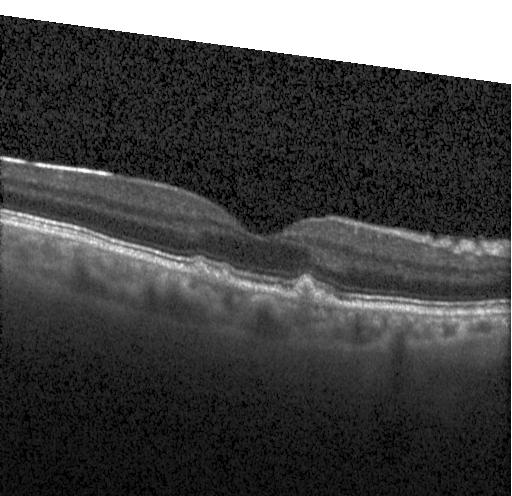
OCT B-scan.
Finding: sub-RPE drusenoid deposits.